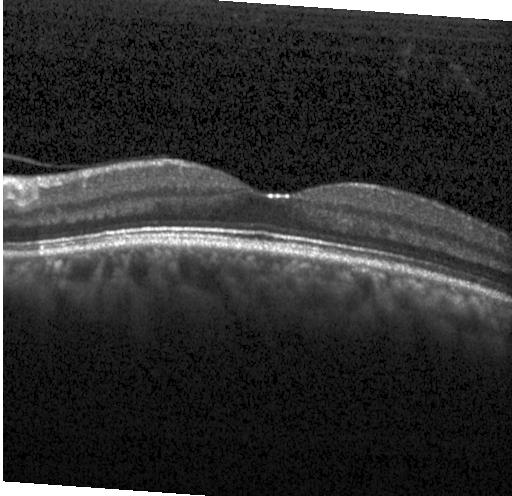

Spectral-domain optical coherence tomography · fovea-centered · optical coherence tomography scan · instrument: Heidelberg Spectralis.
Assessment: no choroidal neovascularization, diabetic macular edema, or drusen.